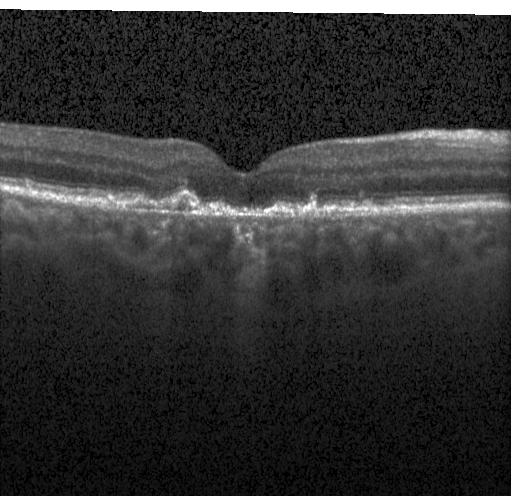 Retinal OCT B-scan · Heidelberg Spectralis OCT system · spectral-domain optical coherence tomography — Impression: a choroidal neovascular membrane.